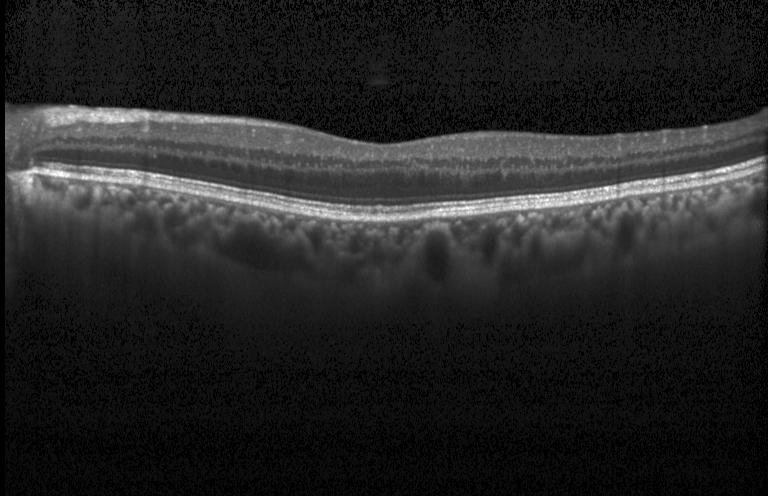 This B-scan demonstrates neither choroidal neovascularization, diabetic macular edema, nor drusen.